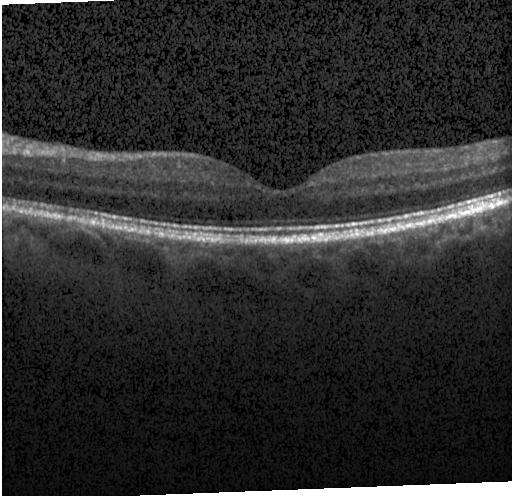

Dx: no choroidal neovascularization, diabetic macular edema, or drusen.